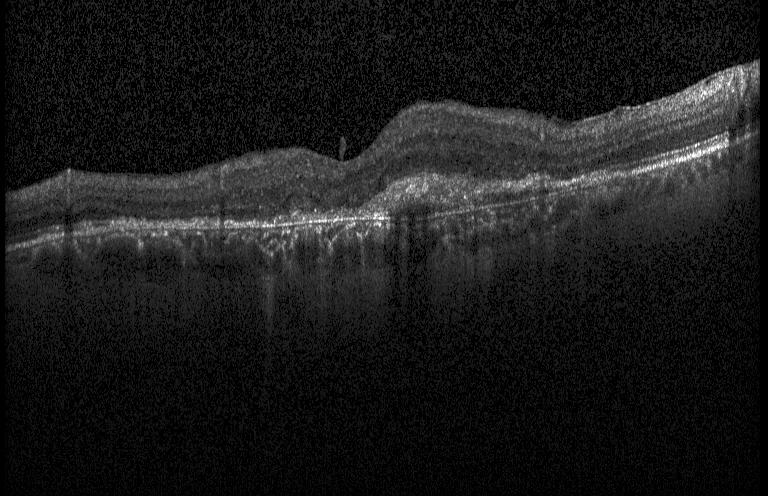
OCT line scan; Heidelberg Spectralis OCT system. Finding: a choroidal neovascular membrane.